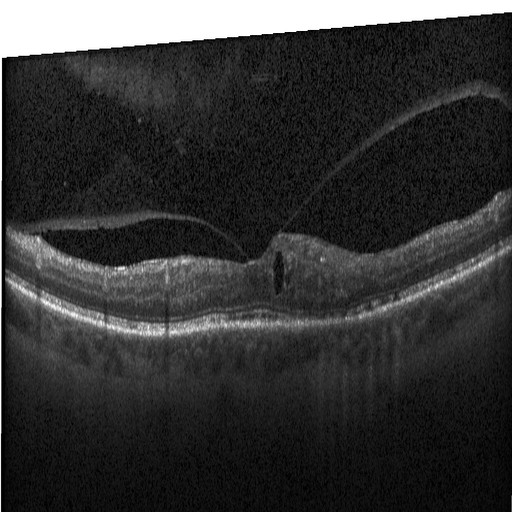 Assessment: diabetic macular edema.